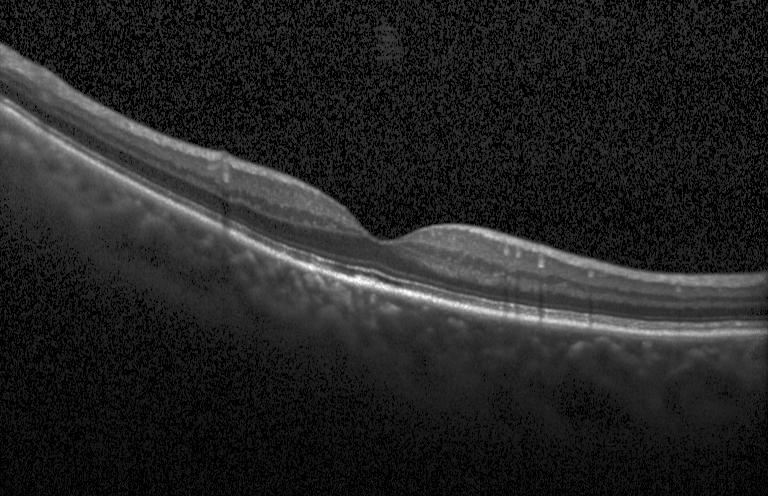 OCT line scan
Dx: neither CNV, DME, nor drusen.